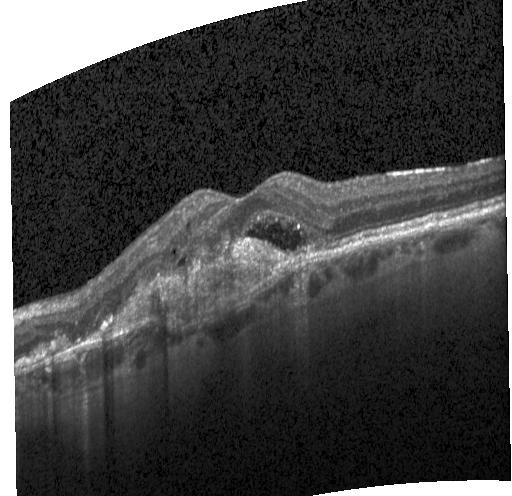

Spectral-domain OCT. Horizontal scan through the fovea. Optical coherence tomography B-scan. Instrument: Heidelberg Spectralis. Diagnosis: choroidal neovascularization.